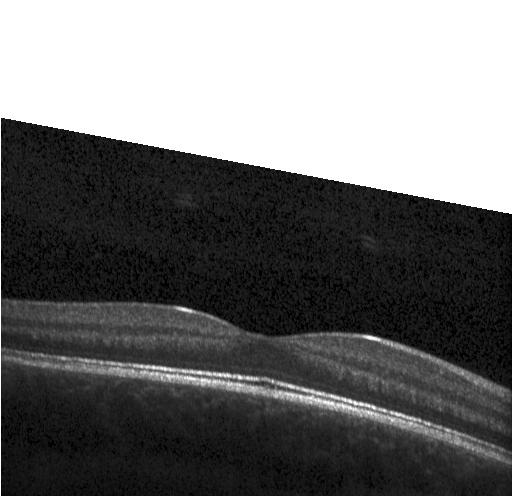

Horizontal scan through the fovea; Heidelberg Spectralis OCT system; OCT line scan; SD-OCT.
Assessment: no evidence of choroidal neovascularization, diabetic macular edema, or drusen.